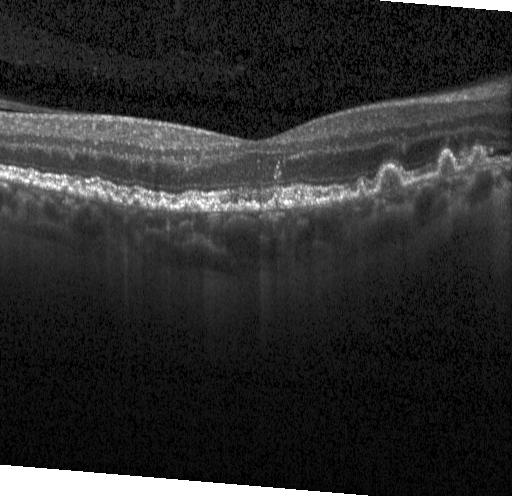
Macular OCT: CNV.